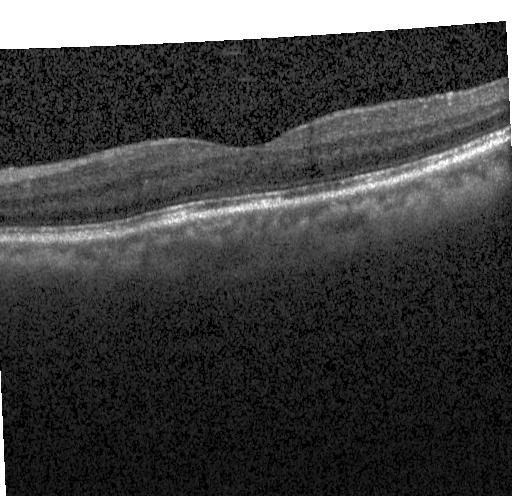 Finding: no evidence of CNV, DME, or drusen.